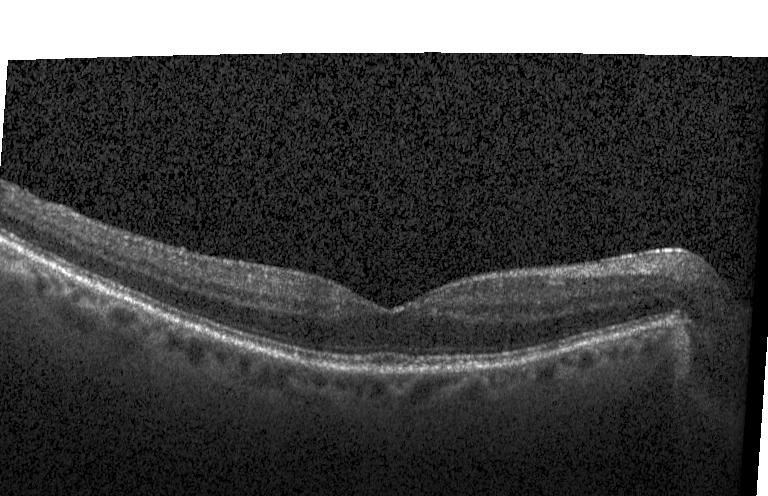

Retinal OCT B-scan · fovea-centered. The scan shows neither choroidal neovascularization, diabetic macular edema, nor drusen.